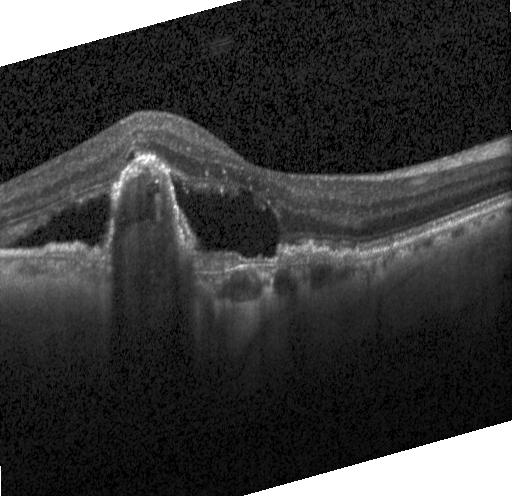

Retinal OCT cross-section.
Diagnosis: a choroidal neovascular membrane.